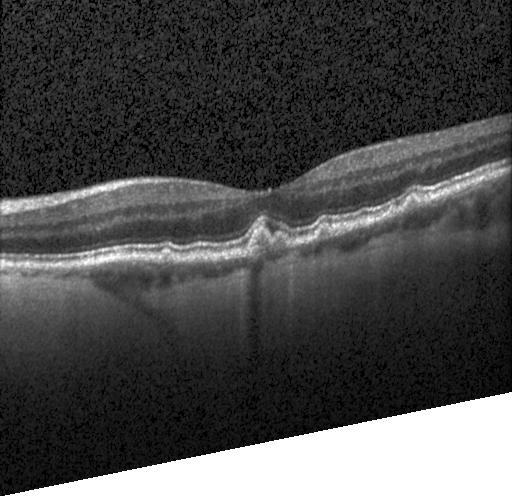 Diagnosis: multiple drusen.